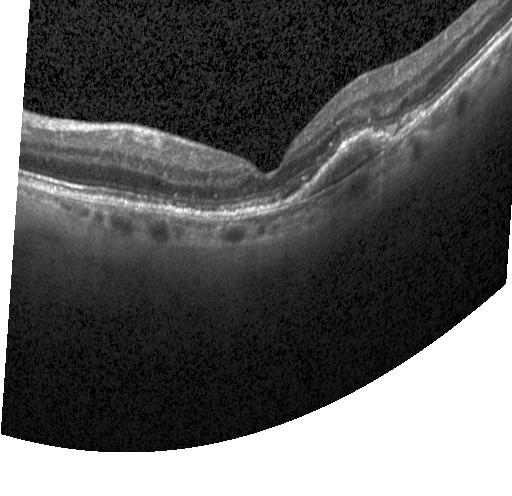 Diagnosis: a choroidal neovascular membrane.